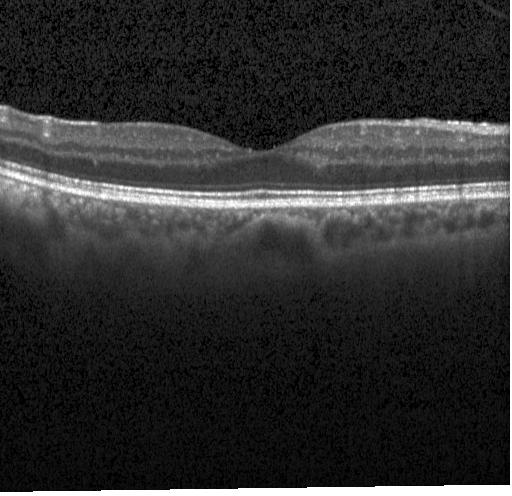

Spectral-domain OCT B-scan: no choroidal neovascularization, diabetic macular edema, or drusen.